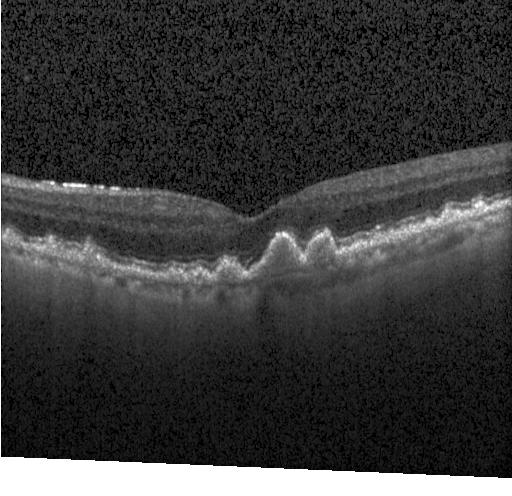
OCT B-scan showing multiple drusen.